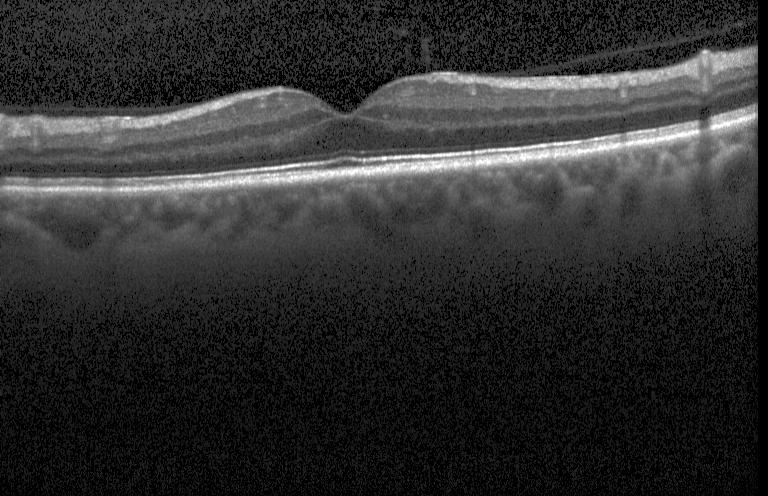 Centered on the fovea · optical coherence tomography B-scan · spectral-domain optical coherence tomography — Diagnosis: no choroidal neovascularization, no diabetic macular edema, and no drusen.